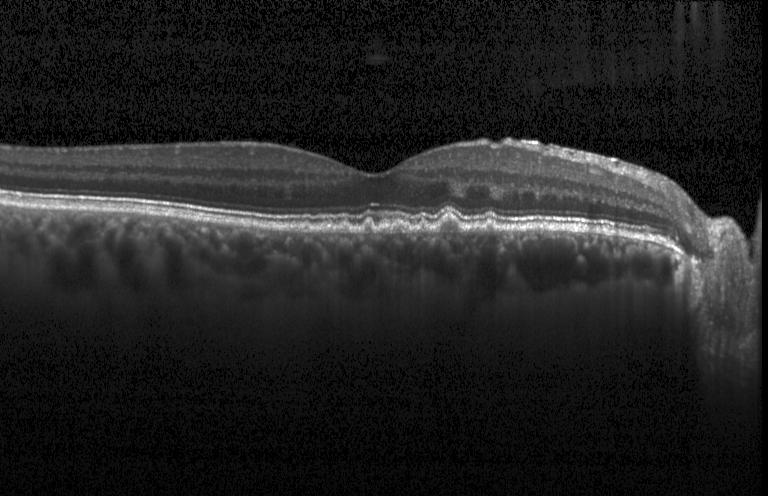
SD-OCT, retinal OCT B-scan — Diagnosis: multiple drusen.